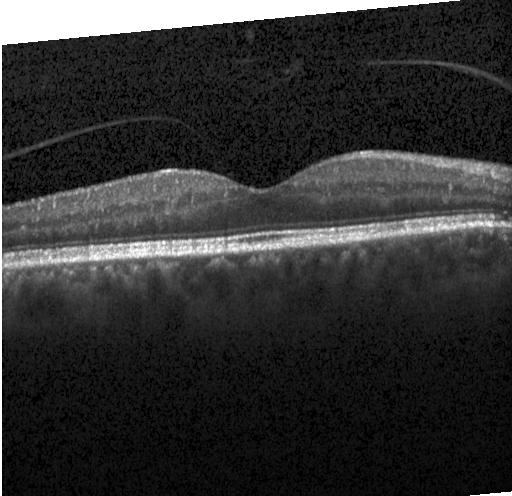 Finding: no CNV, DME, or drusen.